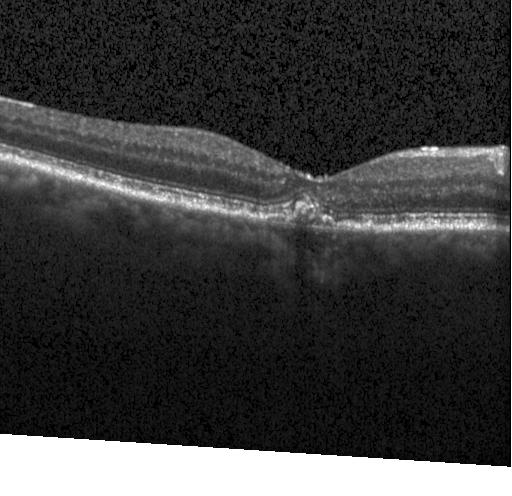 Heidelberg Spectralis OCT system · optical coherence tomography scan
Finding: sub-RPE drusenoid deposits.